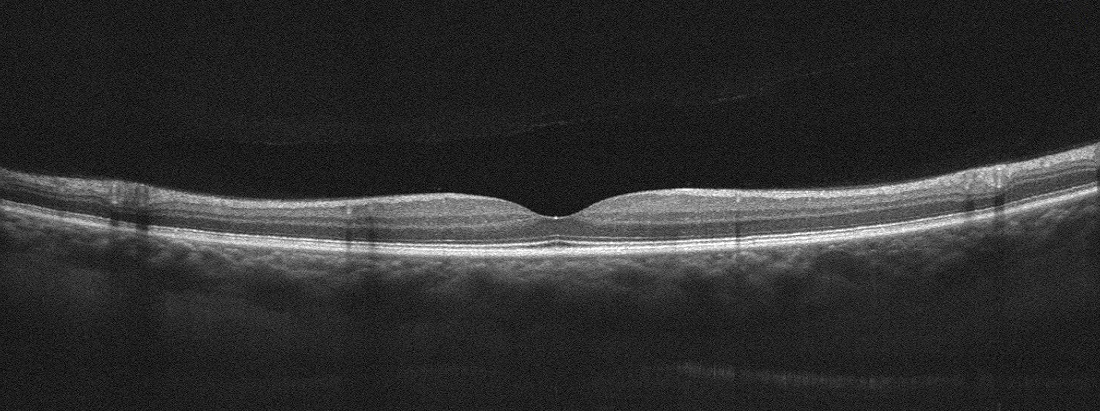 Impression: no evidence of AMD, DME, ERM, RAO, RVO, or VID.